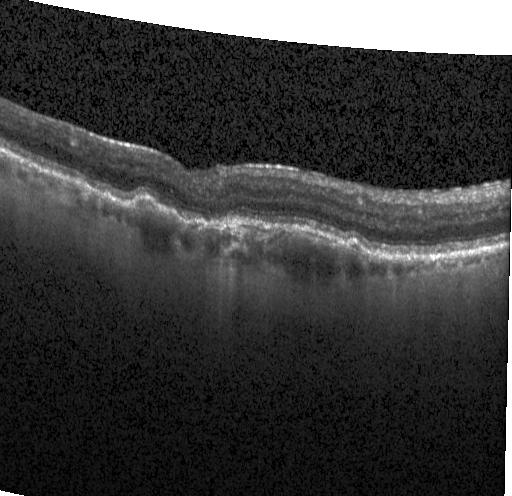

Retinal OCT cross-section
Macular OCT: a choroidal neovascular membrane.